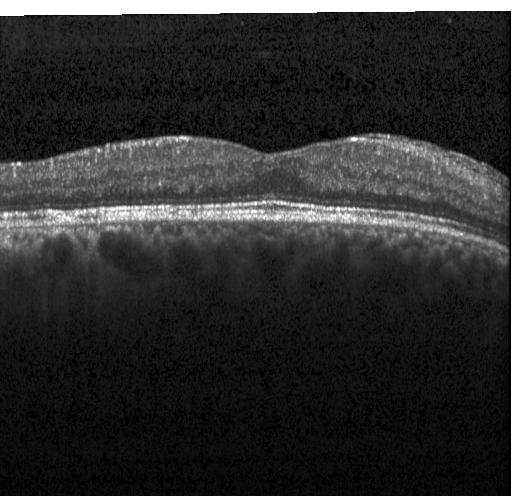

Finding: no CNV, no DME, and no drusen.